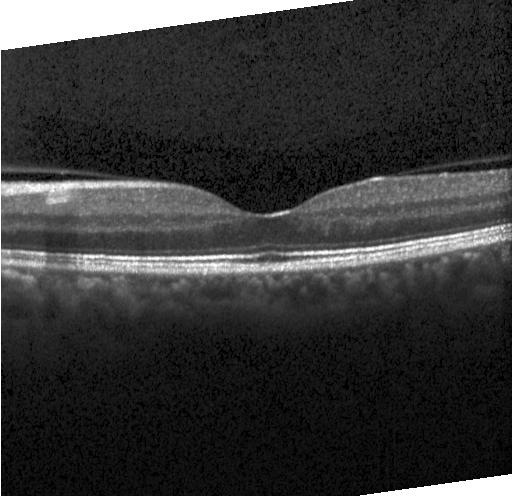 Retinal OCT B-scan; centered on the fovea; spectral-domain OCT; Heidelberg Spectralis. Finding: no evidence of choroidal neovascularization, diabetic macular edema, or drusen.